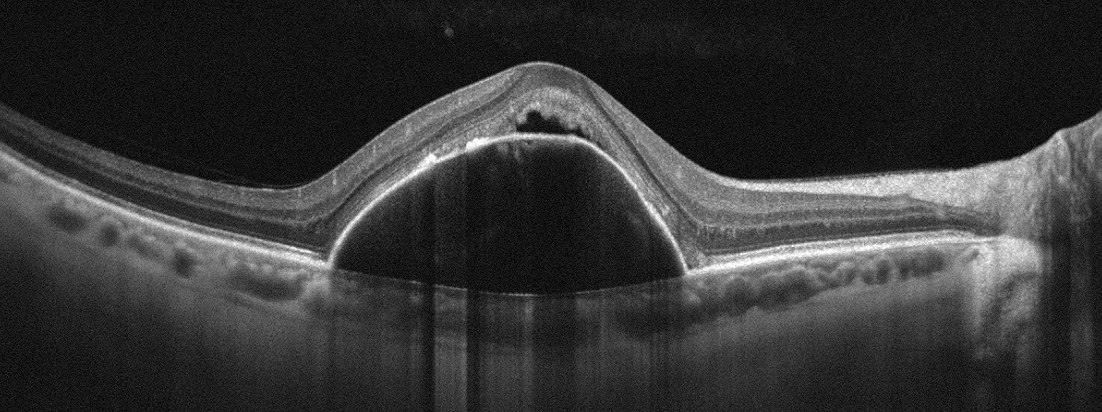
Macular scan. Optovue Avanti RTVue XR. OCT line scan
OCT finding: age-related macular degeneration.